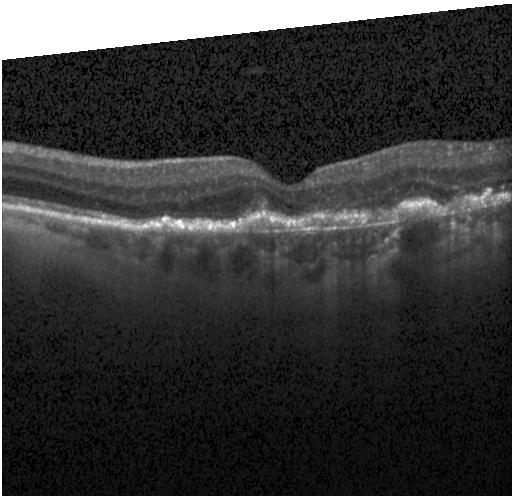

Horizontal scan through the fovea · SD-OCT · optical coherence tomography B-scan.
Finding: a choroidal neovascular membrane.